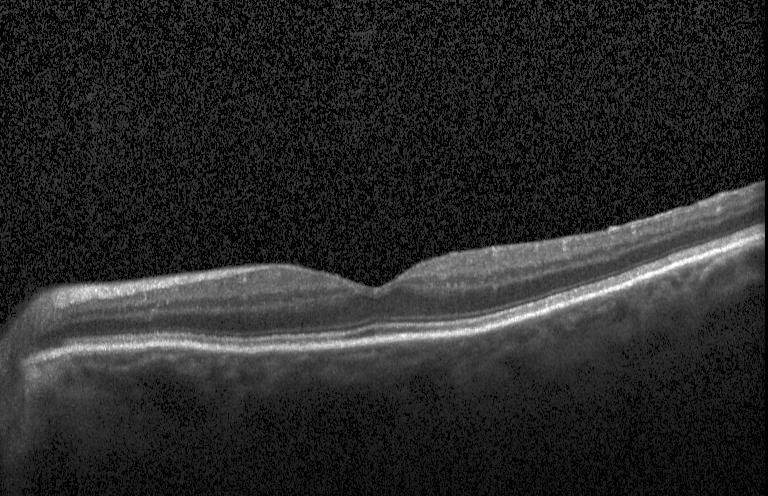 Retinal OCT B-scan, Heidelberg Spectralis — The scan shows no choroidal neovascularization, no diabetic macular edema, and no drusen.